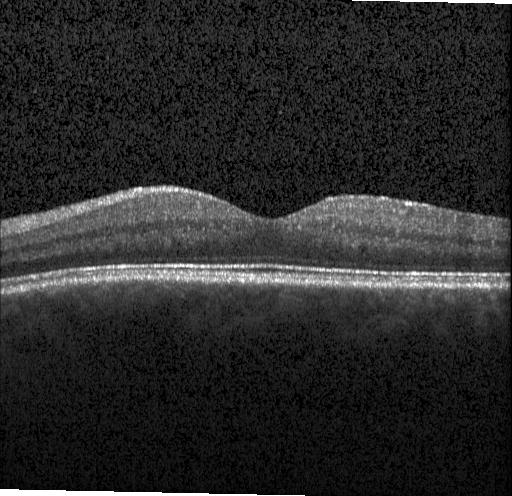

OCT line scan — Diagnosis: no CNV, no DME, and no drusen.